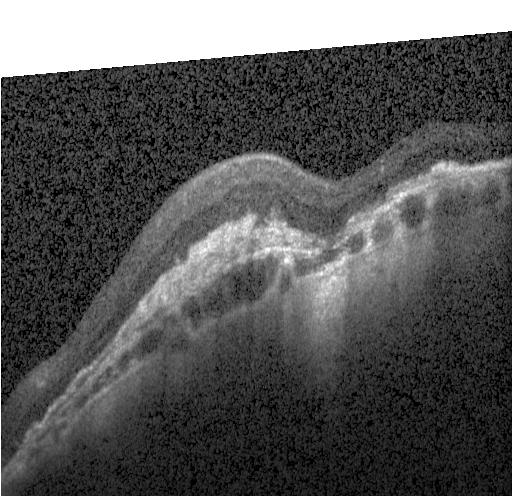
OCT scan showing choroidal neovascularization (CNV).